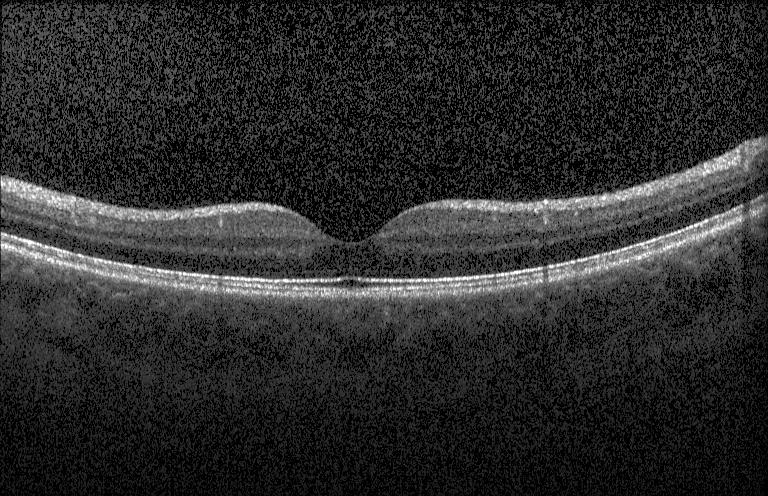

Spectral-domain OCT B-scan: neither choroidal neovascularization, diabetic macular edema, nor drusen.